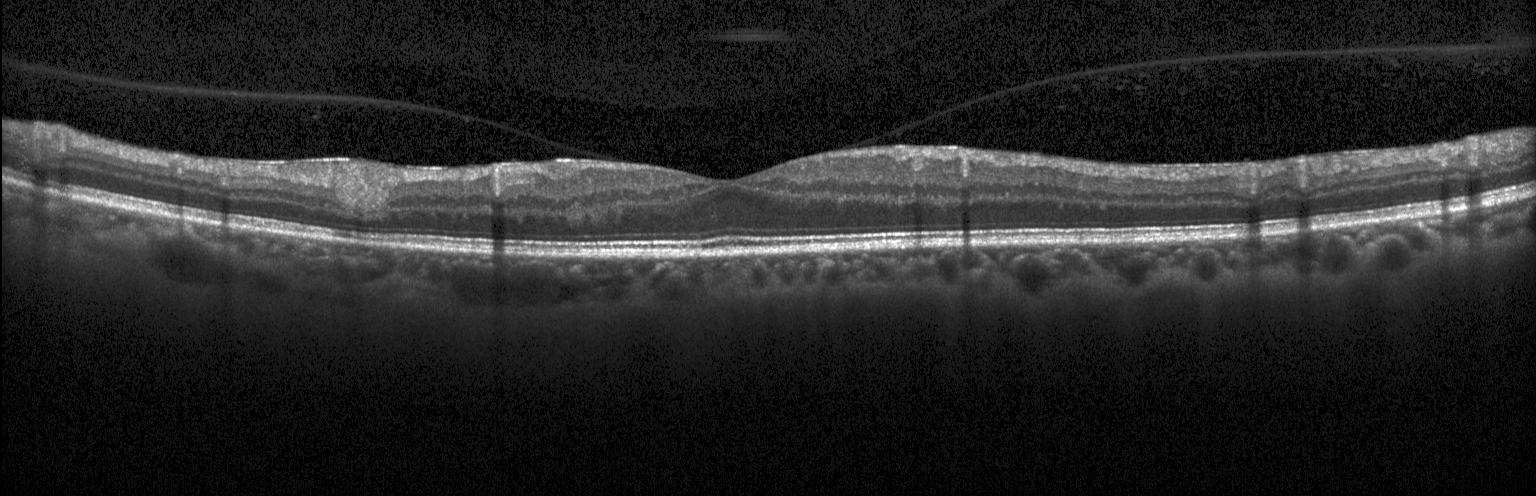 OCT finding: no evidence of CNV, DME, or drusen.